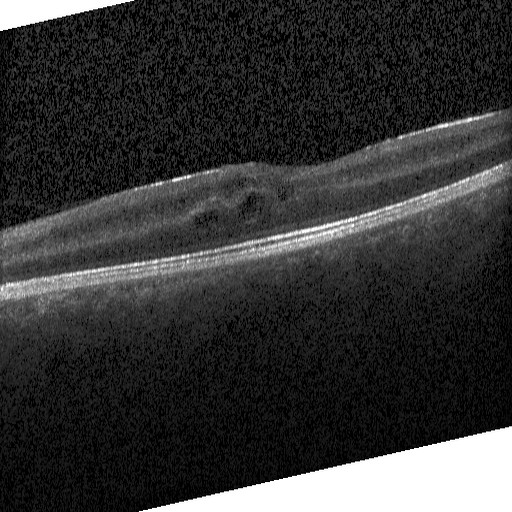 Spectral-domain OCT · OCT line scan. Dx: diabetic macular edema (DME).